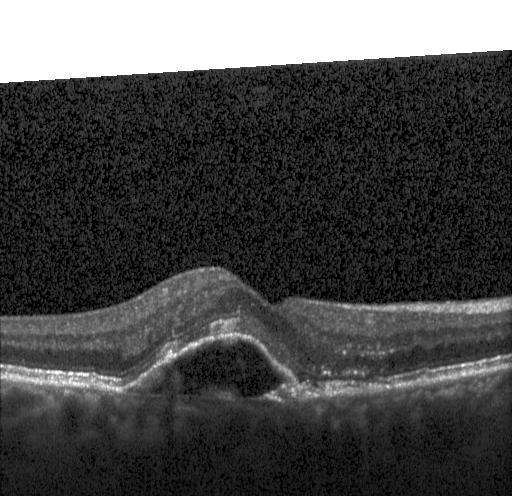 Spectral-domain OCT B-scan: a choroidal neovascular membrane.